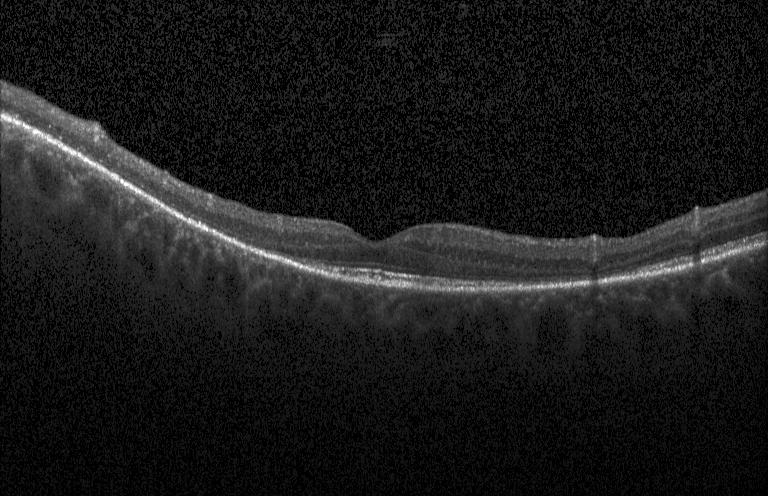

No choroidal neovascularization, no diabetic macular edema, and no drusen.